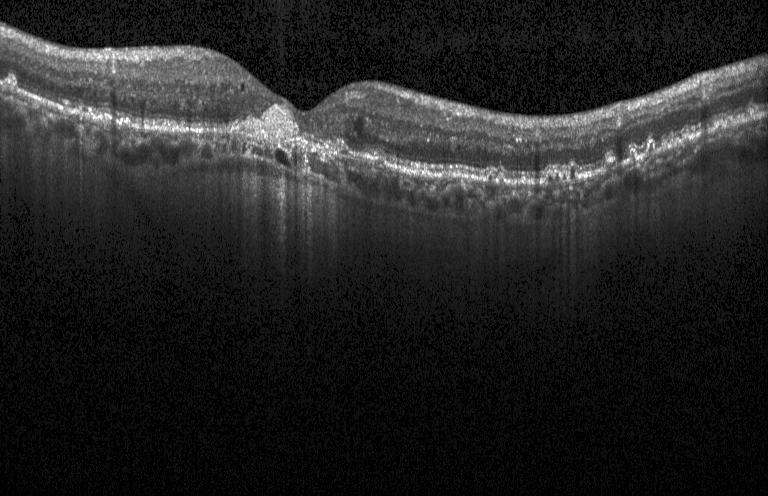
Macular OCT: a choroidal neovascular membrane.